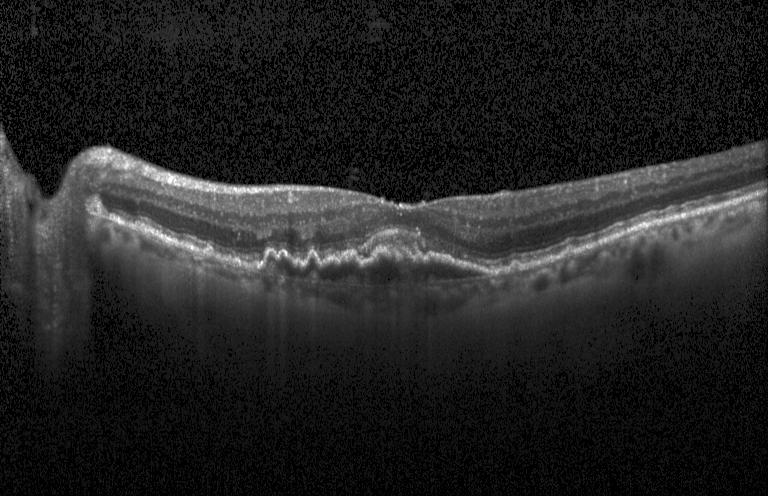

A choroidal neovascular membrane.